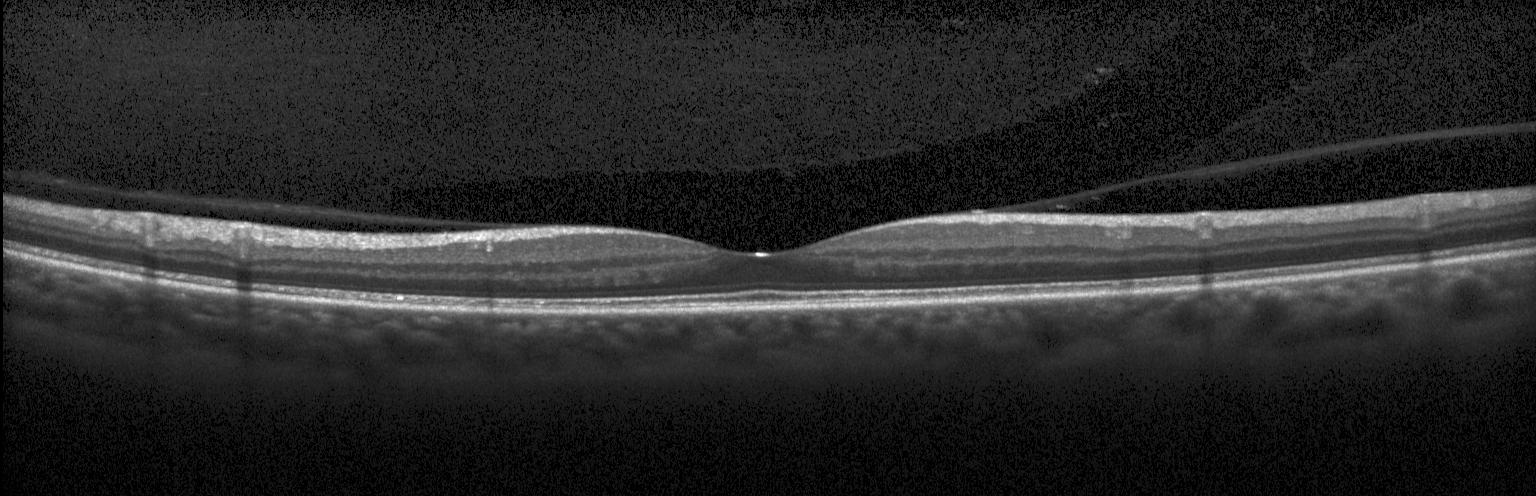
OCT line scan. Fovea-centered. Acquired on a Heidelberg Spectralis — This B-scan demonstrates neither choroidal neovascularization, diabetic macular edema, nor drusen.